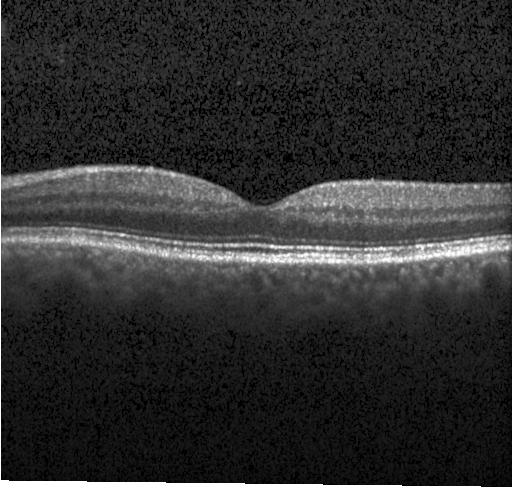
Retinal OCT B-scan. Impression: no choroidal neovascularization, no diabetic macular edema, and no drusen.